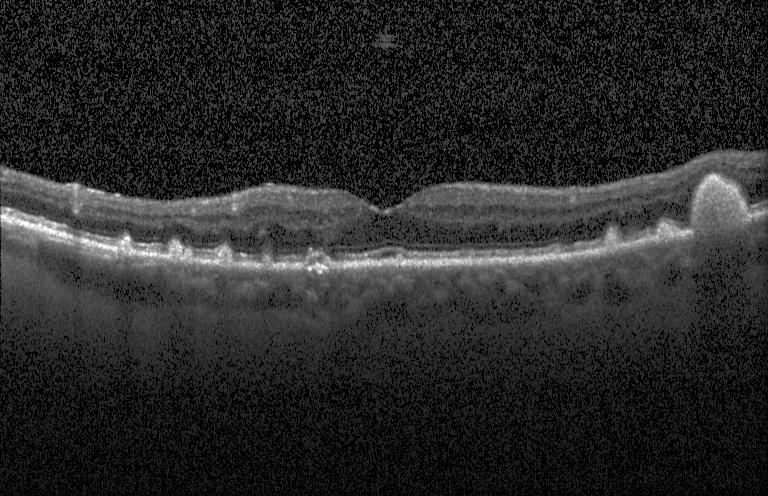 OCT B-scan.
Finding: sub-RPE drusenoid deposits.